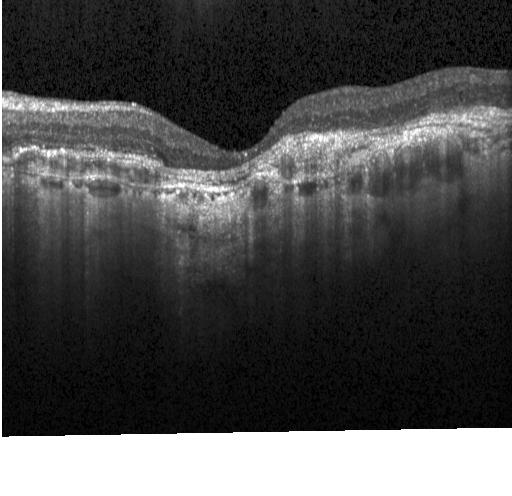

Dx: a choroidal neovascular membrane.